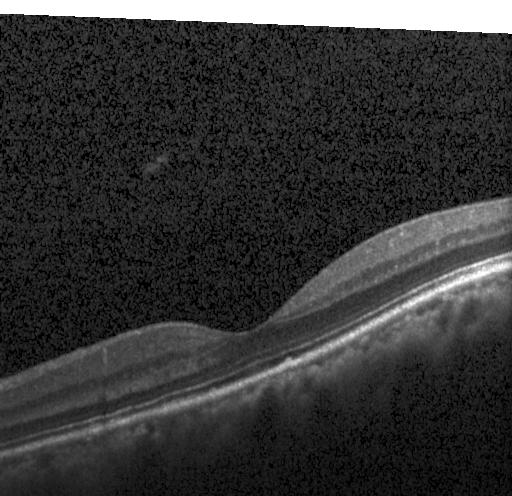 Macular scan · OCT line scan · spectral-domain optical coherence tomography · acquired on a Heidelberg Spectralis — Dx: no CNV, no DME, and no drusen.